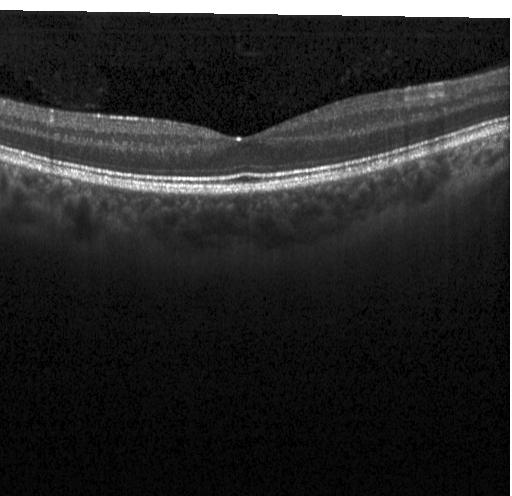

Spectral-domain OCT B-scan: no choroidal neovascularization, diabetic macular edema, or drusen.